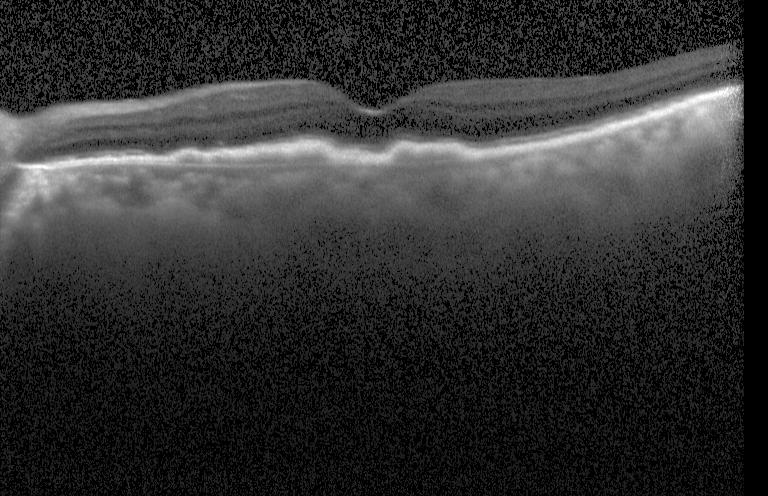
The scan shows CNV.